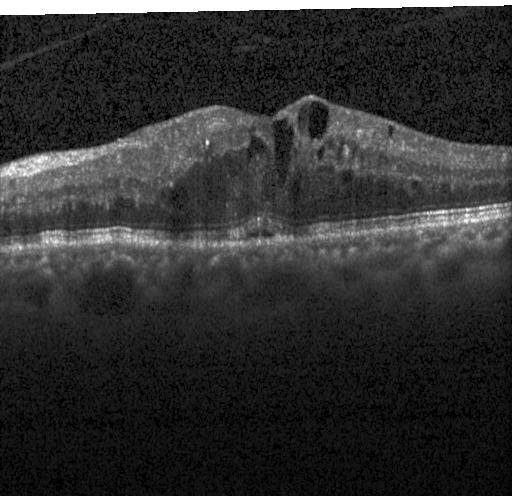
Optical coherence tomography B-scan, spectral-domain OCT, fovea-centered — Impression: diabetic macular edema (DME).